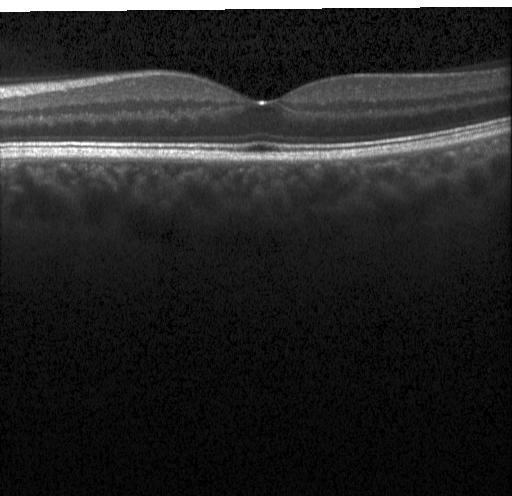
Retinal OCT B-scan.
Macular OCT: no CNV, no DME, and no drusen.